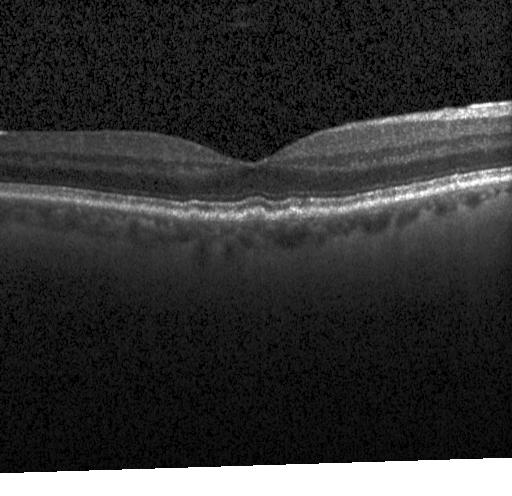
Finding: sub-RPE drusenoid deposits.